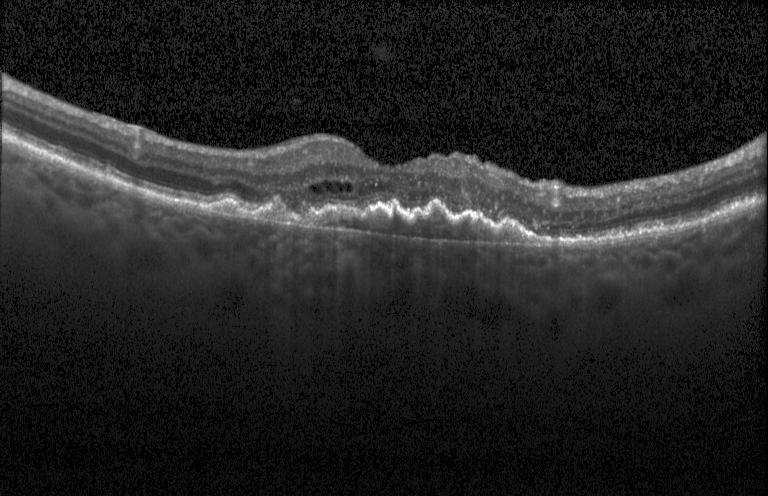
Diagnosis: a choroidal neovascular membrane.